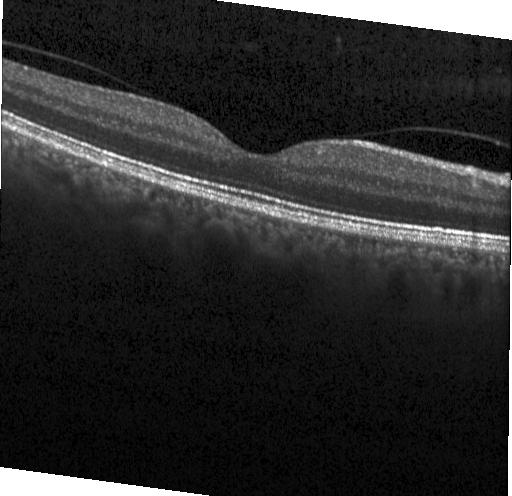 Acquired on a Heidelberg Spectralis. Spectral-domain optical coherence tomography. Horizontal scan through the fovea. Optical coherence tomography scan — Diagnosis: no evidence of choroidal neovascularization, diabetic macular edema, or drusen.